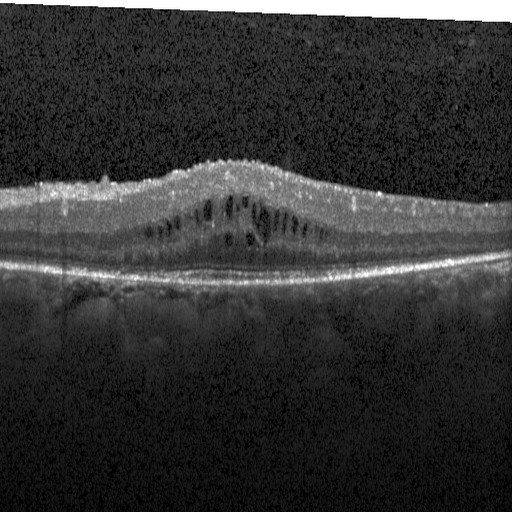

Heidelberg Spectralis · optical coherence tomography scan. Diagnosis: diabetic macular edema.